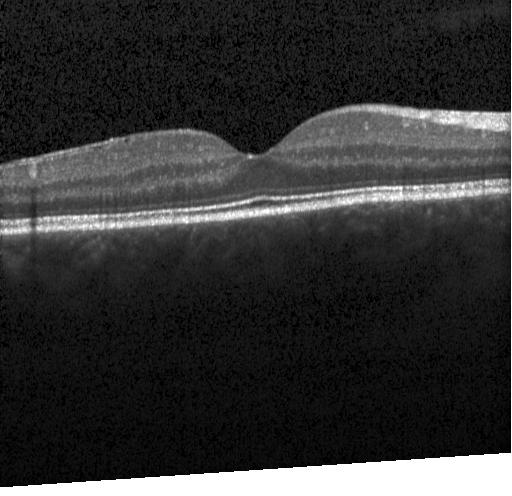

Retinal OCT B-scan
Diagnosis: no choroidal neovascularization, diabetic macular edema, or drusen.